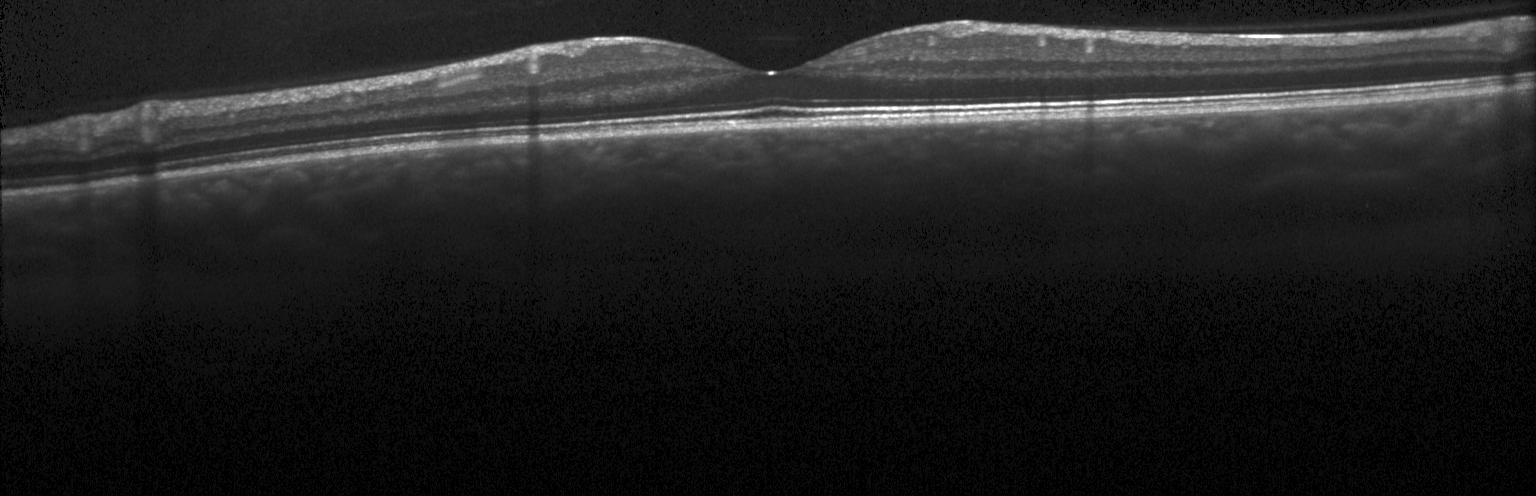 Dx: no choroidal neovascularization, diabetic macular edema, or drusen.